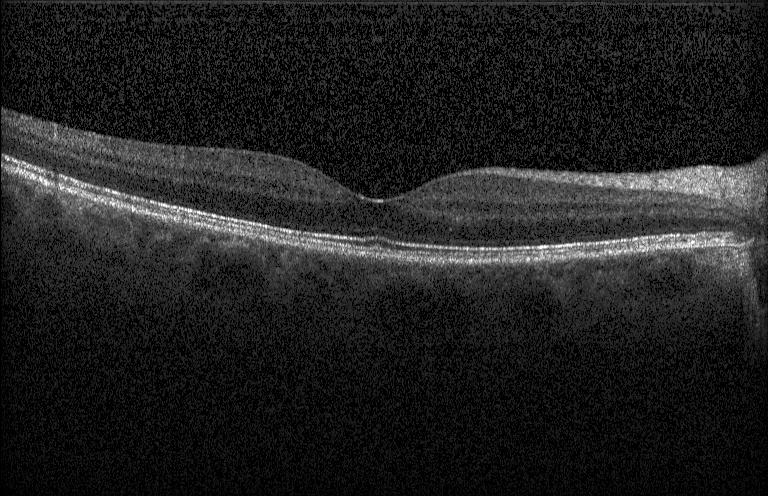
SD-OCT; optical coherence tomography B-scan; fovea-centered — OCT finding: no CNV, DME, or drusen.